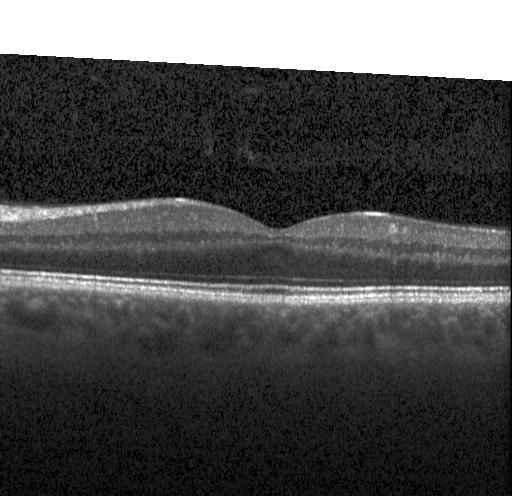 Diagnosis: no choroidal neovascularization, no diabetic macular edema, and no drusen.